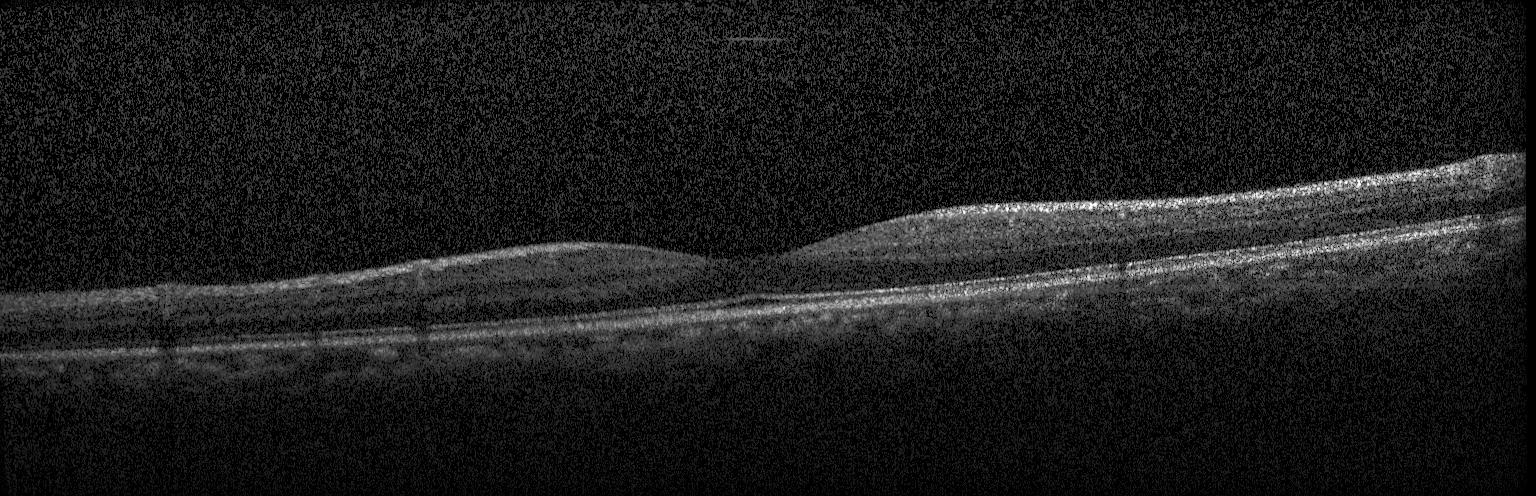
Optical coherence tomography B-scan; instrument: Heidelberg Spectralis; through the macula
Finding: no evidence of choroidal neovascularization, diabetic macular edema, or drusen.